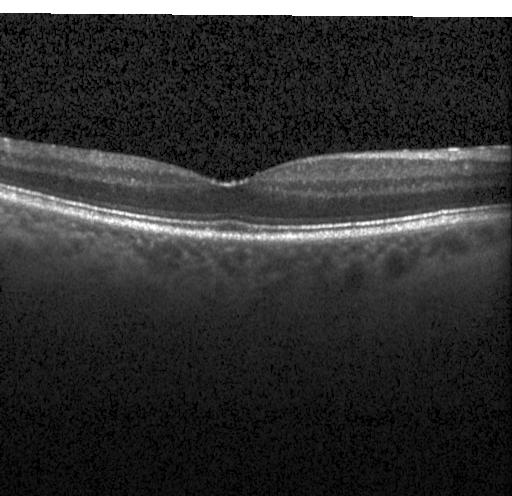

Finding: neither choroidal neovascularization, diabetic macular edema, nor drusen.